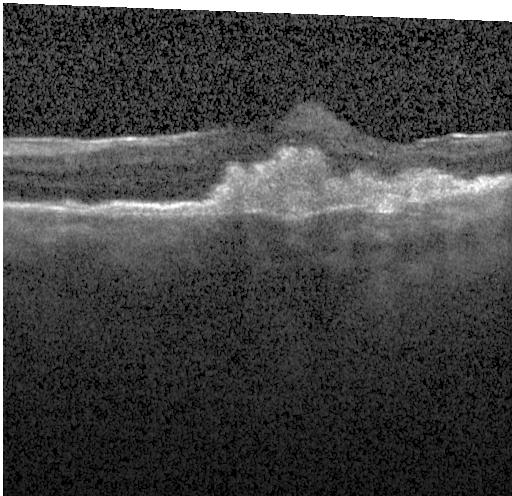
OCT line scan.
Finding: a choroidal neovascular membrane.